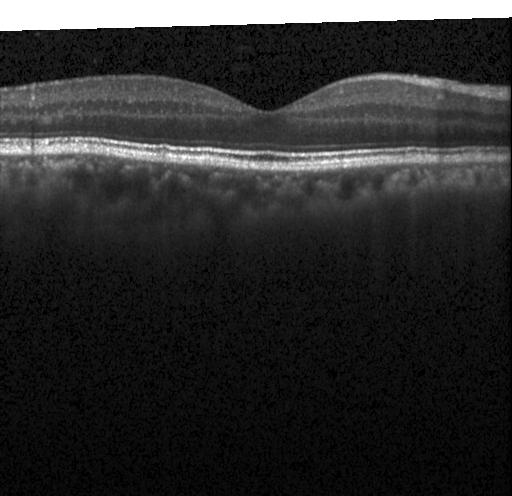 Diagnosis: no choroidal neovascularization, diabetic macular edema, or drusen.